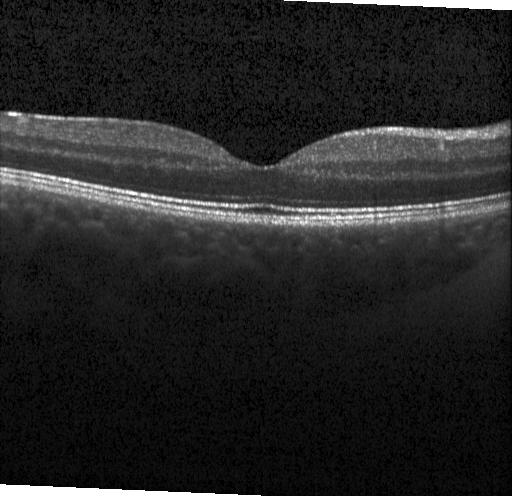
Optical coherence tomography scan, spectral-domain optical coherence tomography. Finding: neither choroidal neovascularization, diabetic macular edema, nor drusen.